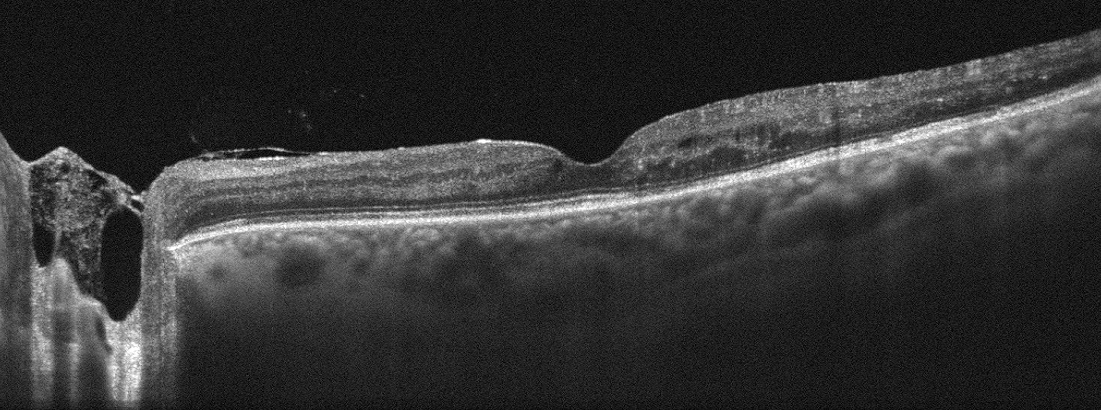 Optical coherence tomography B-scan; macular scan — Finding: diabetic macular edema.